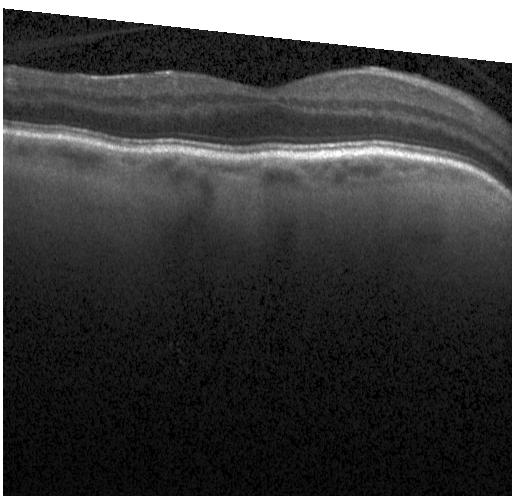

OCT line scan, fovea-centered, spectral-domain OCT, acquired on a Heidelberg Spectralis
Assessment: no CNV, DME, or drusen.